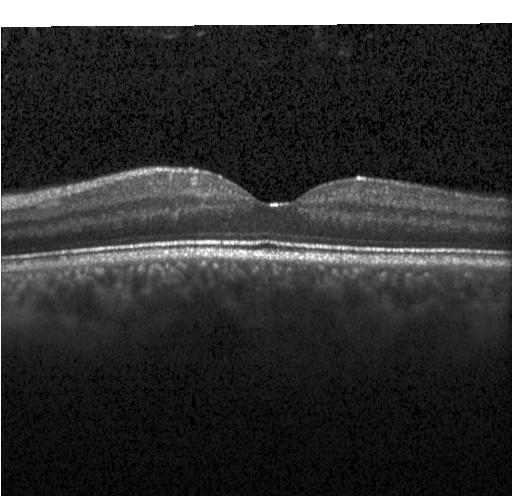
Retinal OCT cross-section showing no CNV, no DME, and no drusen.